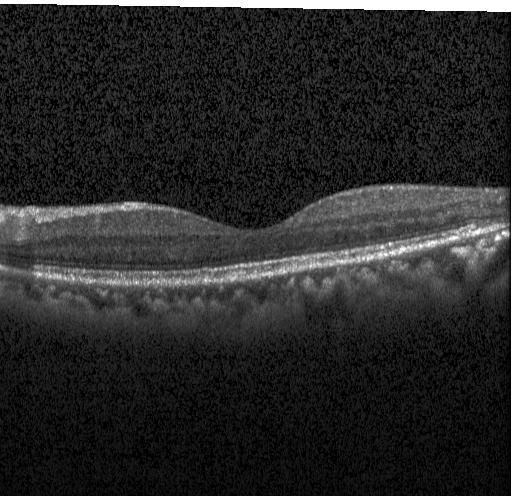

Retinal OCT cross-section. Heidelberg Spectralis. Spectral-domain OCT. Through the macula. This B-scan demonstrates no choroidal neovascularization, diabetic macular edema, or drusen.